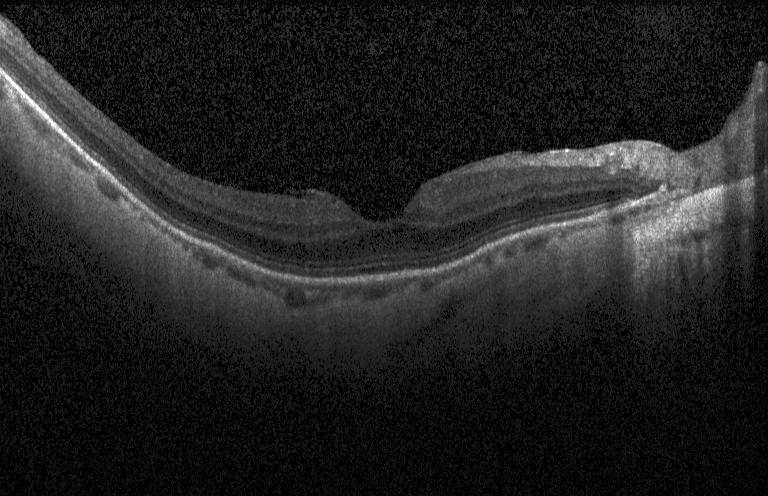 Spectral-domain OCT. Retinal OCT cross-section. Heidelberg Spectralis
Diagnosis: no evidence of choroidal neovascularization, diabetic macular edema, or drusen.